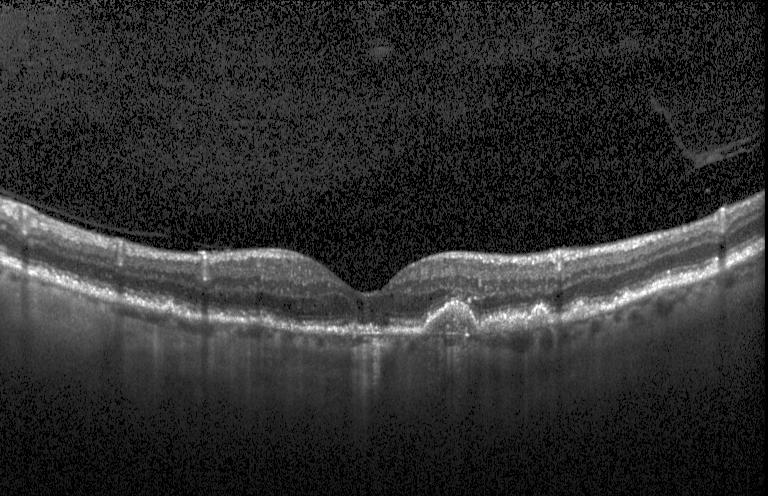
A choroidal neovascular membrane.